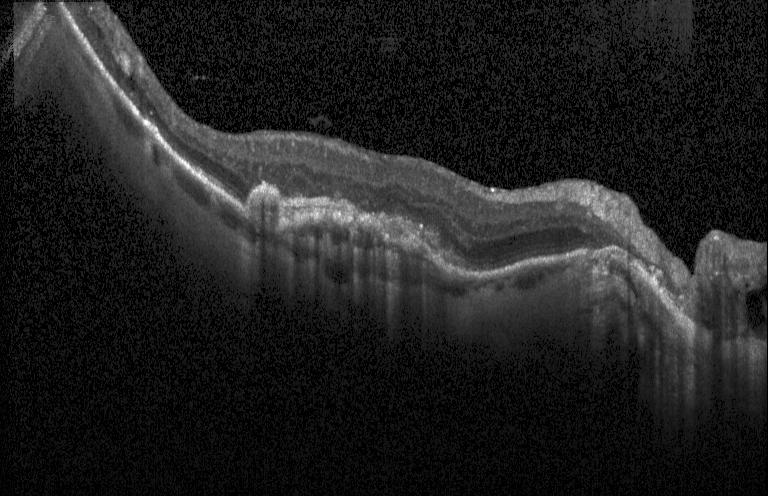 Spectral-domain optical coherence tomography · acquired on a Heidelberg Spectralis · optical coherence tomography scan — Macular OCT: a choroidal neovascular membrane.